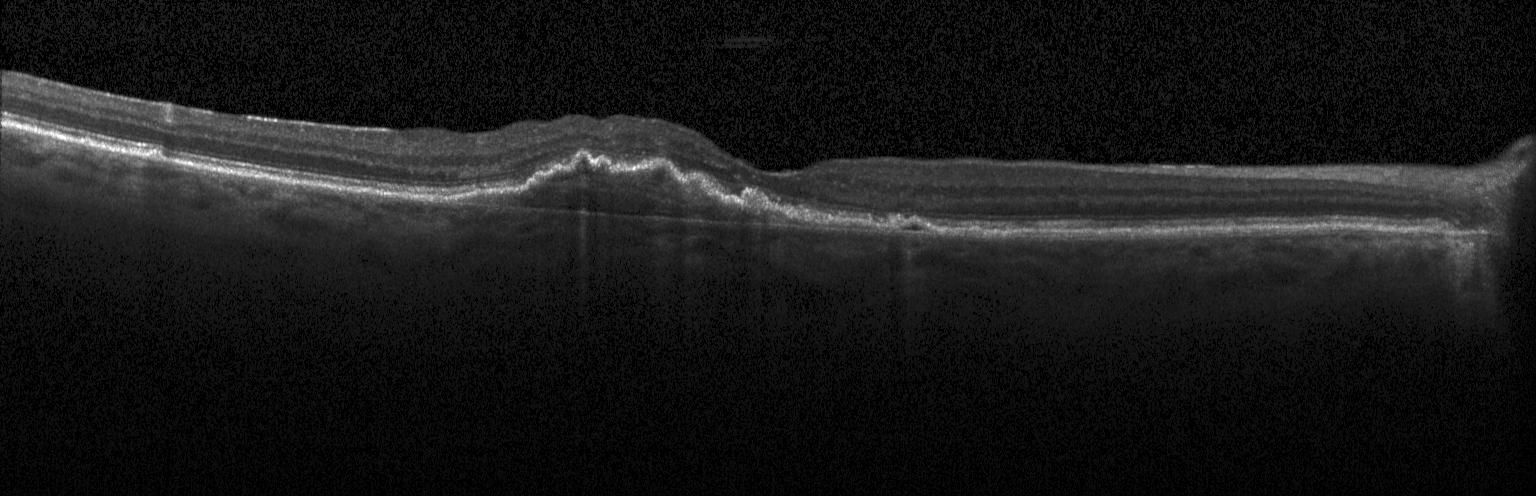

Spectral-domain optical coherence tomography. OCT line scan. Impression: choroidal neovascularization.